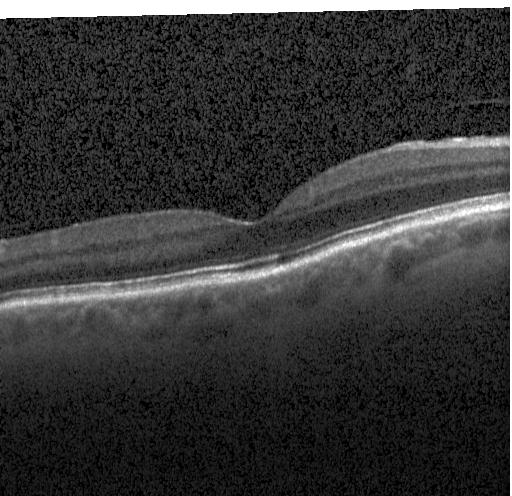
Finding: no CNV, no DME, and no drusen.